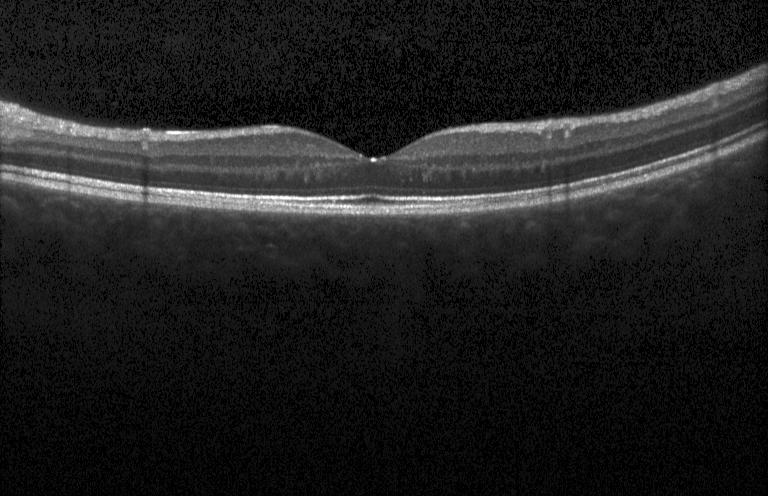 Diagnosis: no choroidal neovascularization, diabetic macular edema, or drusen.